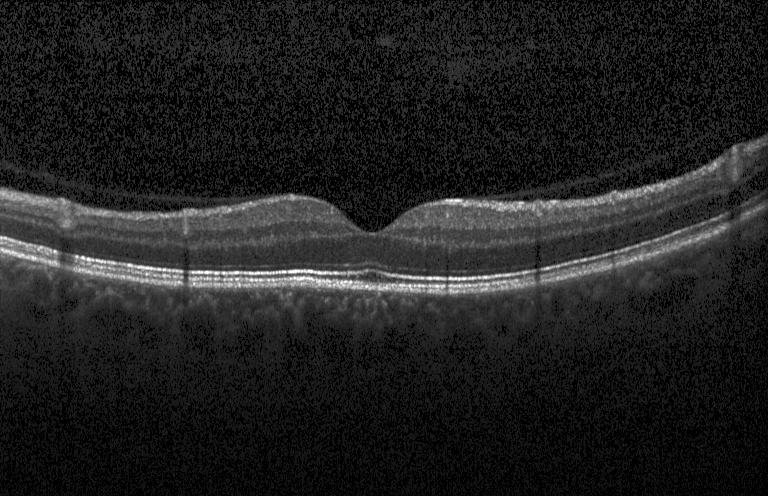 Heidelberg Spectralis, OCT B-scan. Finding: no choroidal neovascularization, no diabetic macular edema, and no drusen.